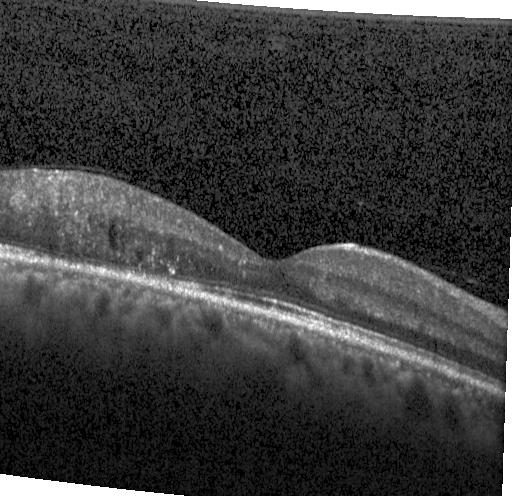

Retinal OCT cross-section. OCT finding: diabetic macular edema.